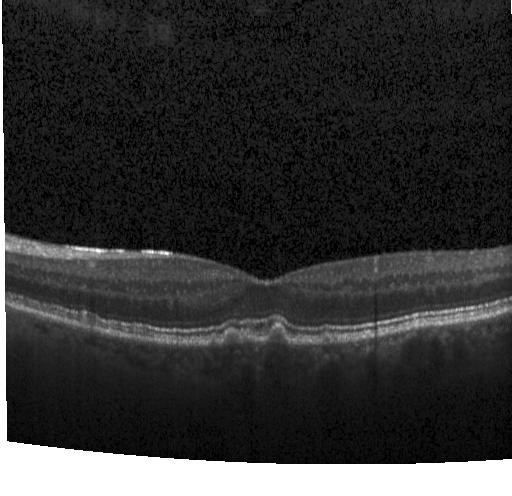 Retinal OCT cross-section showing sub-RPE drusenoid deposits.